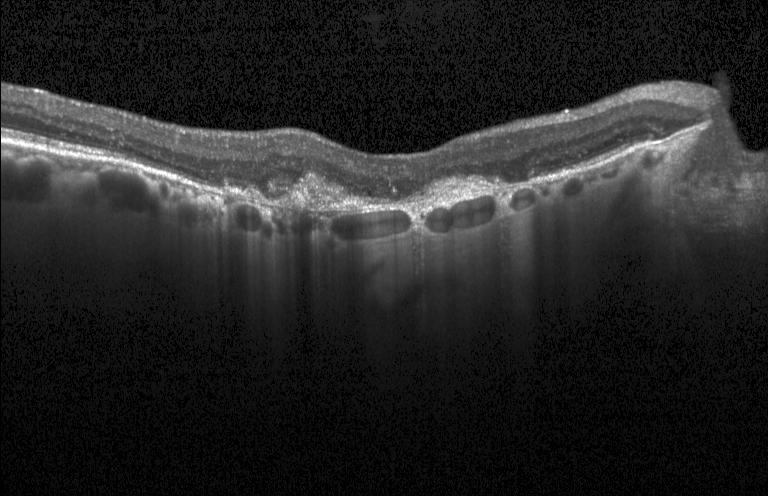

Finding: a choroidal neovascular membrane.